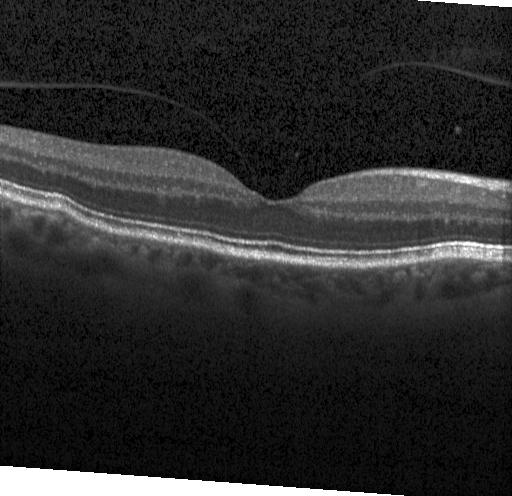
Macular OCT: no choroidal neovascularization, diabetic macular edema, or drusen.